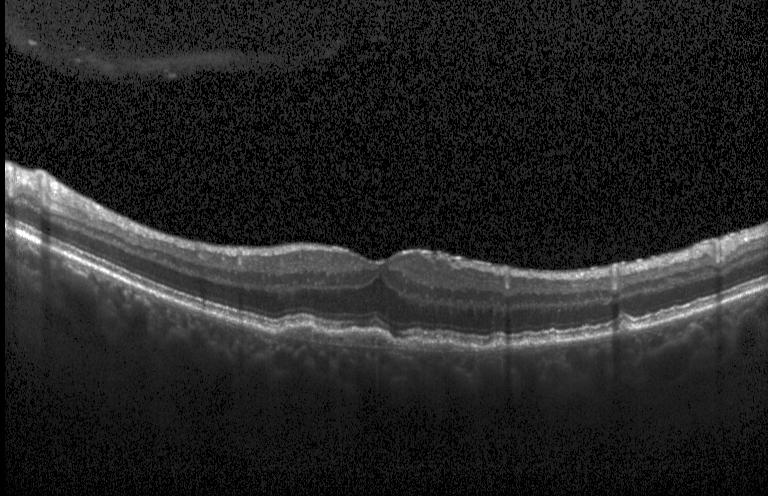
Spectral-domain OCT B-scan: CNV.